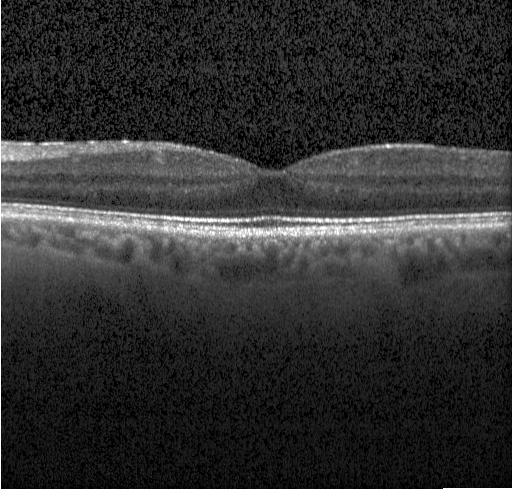 OCT finding: no choroidal neovascularization, diabetic macular edema, or drusen.